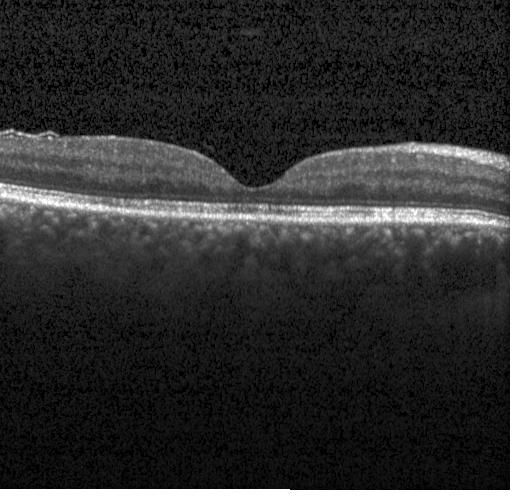

Optical coherence tomography B-scan — The scan shows no evidence of CNV, DME, or drusen.